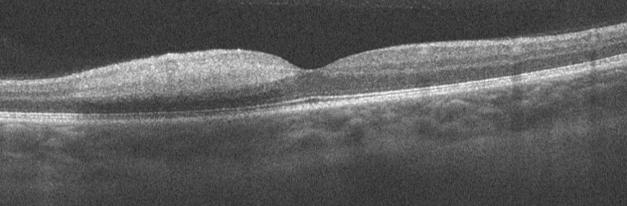 Optical coherence tomography B-scan
Retinal artery occlusion.